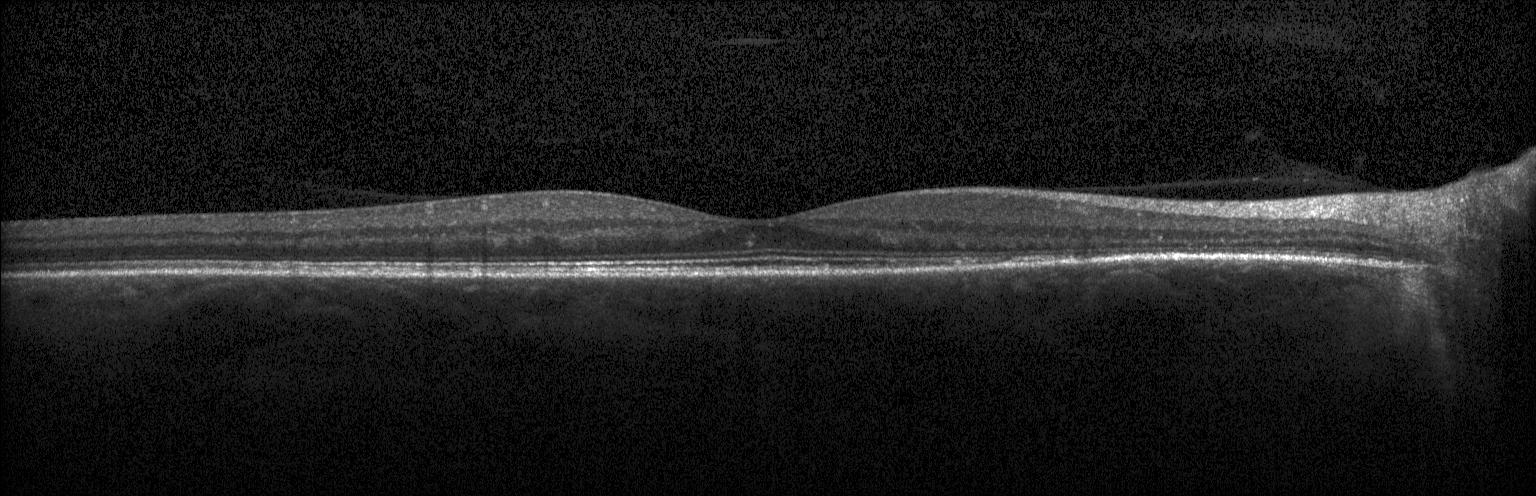
Assessment: no evidence of choroidal neovascularization, diabetic macular edema, or drusen.